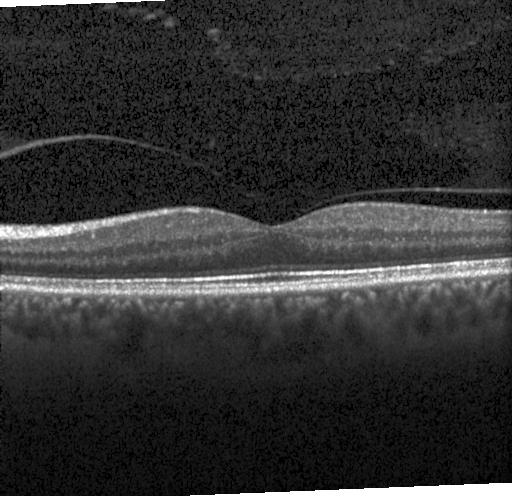
Centered on the fovea; retinal OCT B-scan.
Assessment: no evidence of choroidal neovascularization, diabetic macular edema, or drusen.